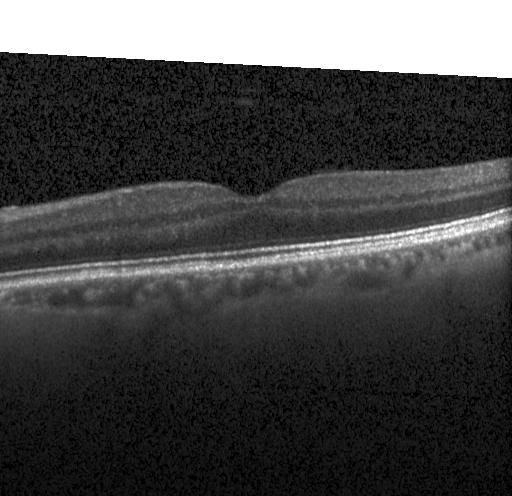

Optical coherence tomography scan. Fovea-centered. Neither choroidal neovascularization, diabetic macular edema, nor drusen.